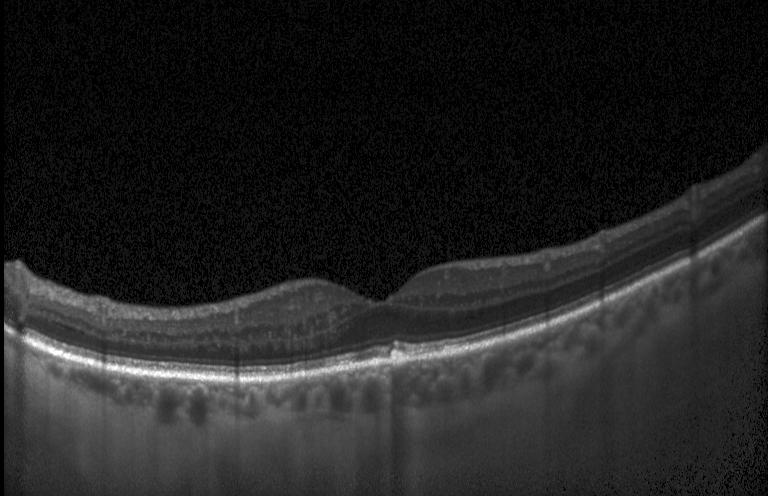
This B-scan demonstrates sub-RPE drusenoid deposits.